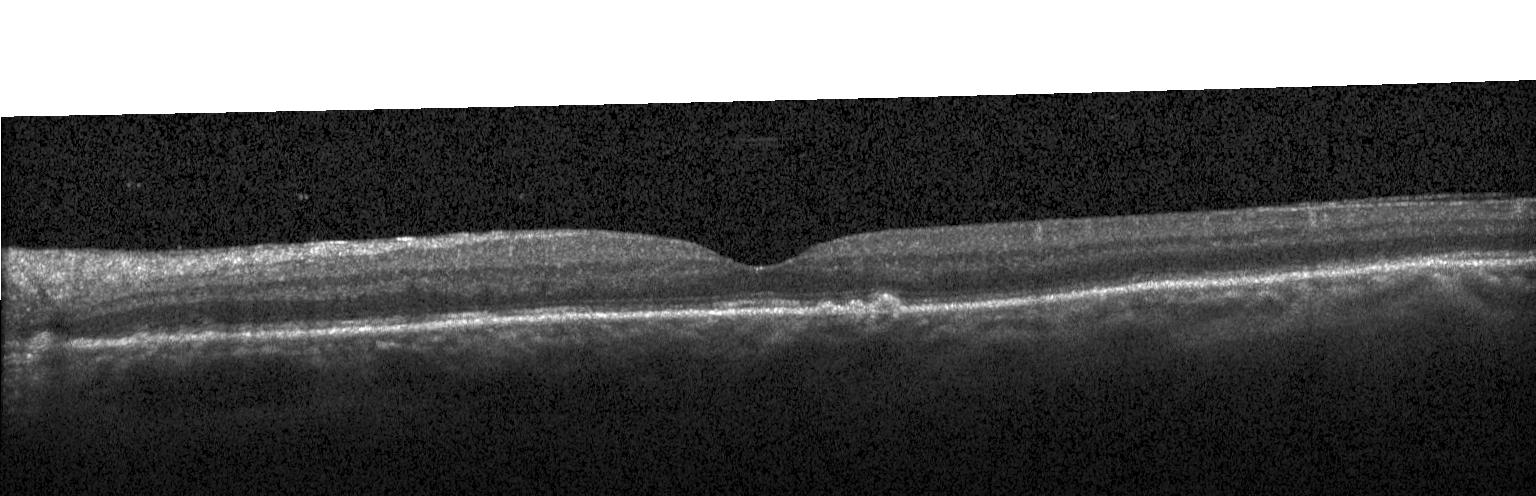

Acquired on a Heidelberg Spectralis; retinal OCT B-scan. This B-scan demonstrates drusen.